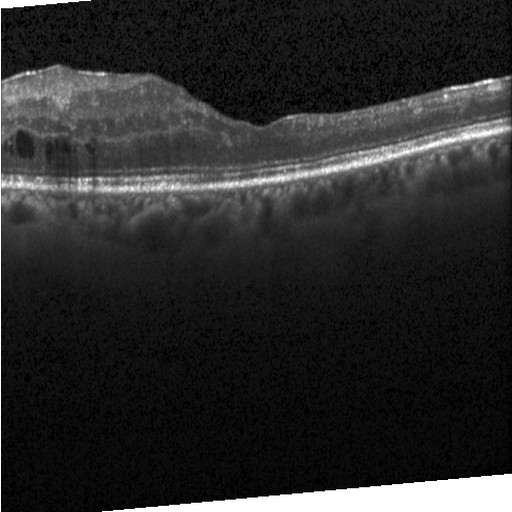
Diagnosis: diabetic macular edema (DME).